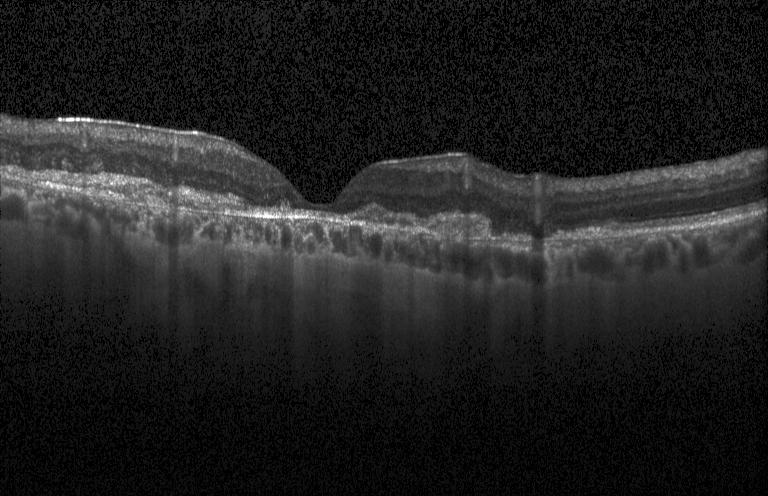

Heidelberg Spectralis · retinal OCT cross-section · SD-OCT
OCT finding: a choroidal neovascular membrane.